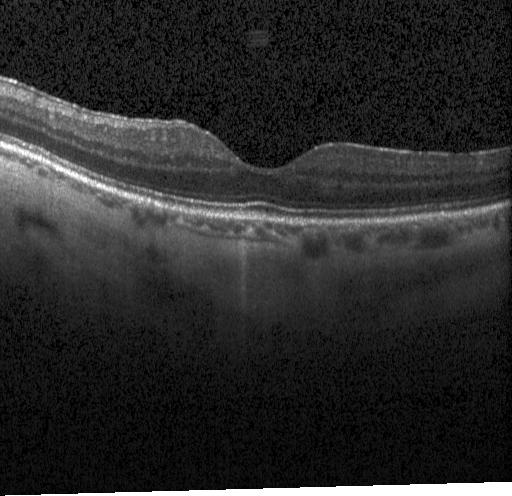

This B-scan demonstrates no evidence of choroidal neovascularization, diabetic macular edema, or drusen.